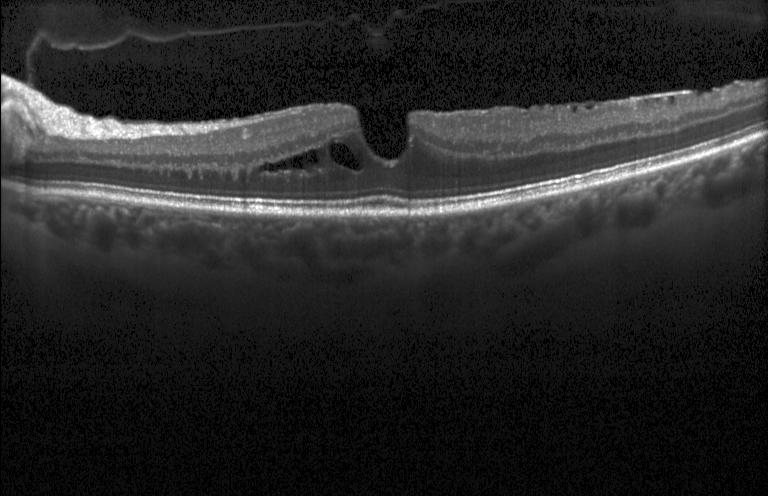 Retinal OCT B-scan; horizontal scan through the fovea — Impression: DME.